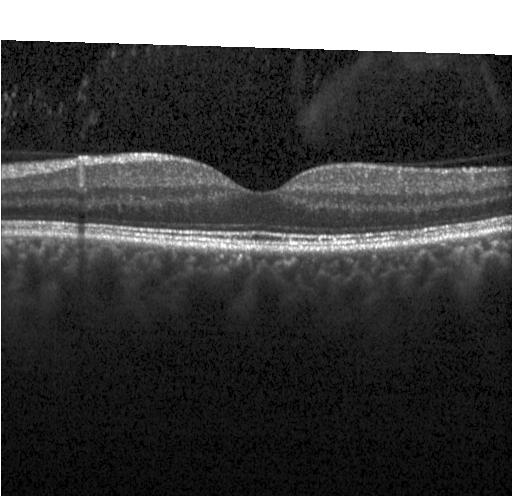 Finding: no choroidal neovascularization, no diabetic macular edema, and no drusen.